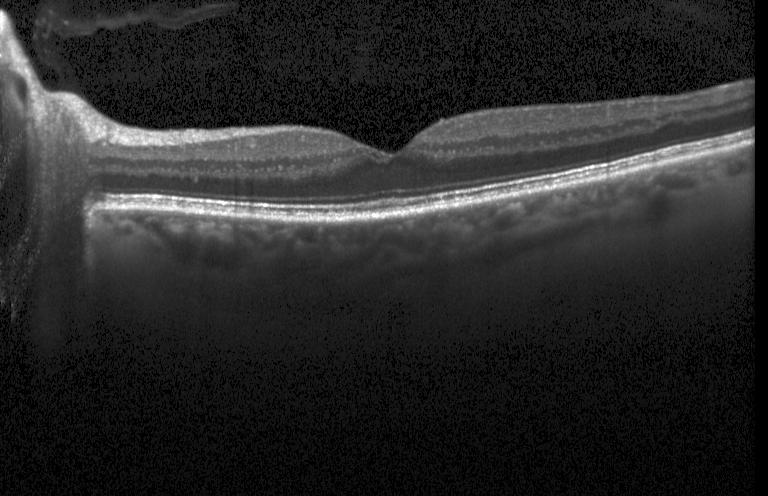
Spectral-domain OCT · OCT B-scan · macular scan · Heidelberg Spectralis OCT system
Finding: no evidence of choroidal neovascularization, diabetic macular edema, or drusen.